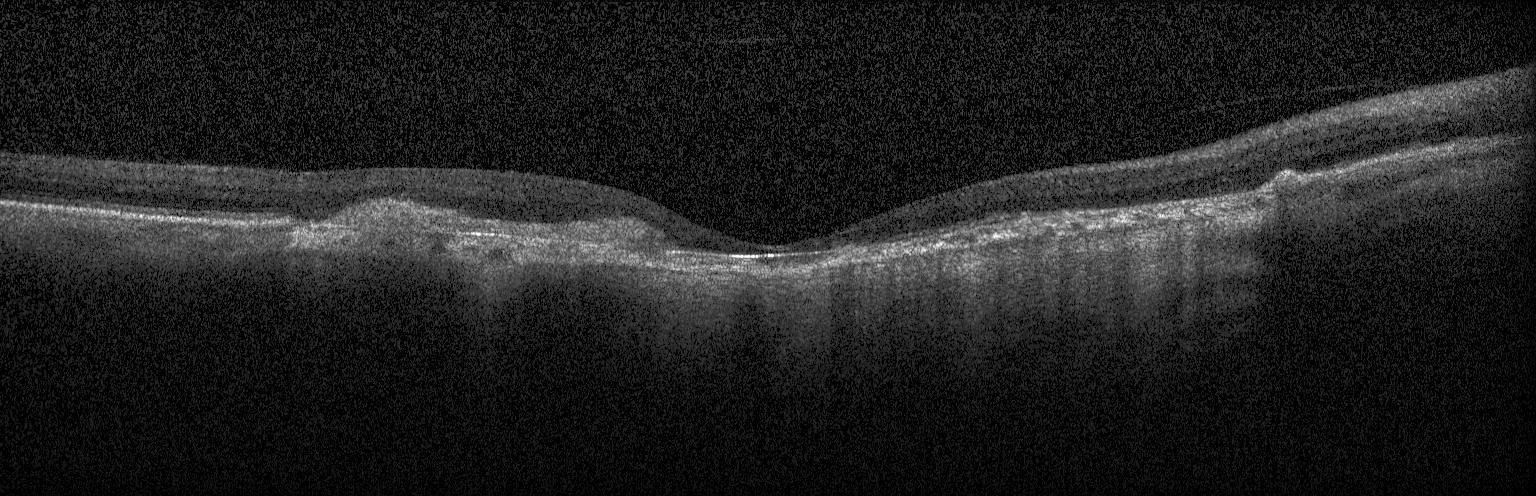
OCT line scan.
This B-scan demonstrates a choroidal neovascular membrane.